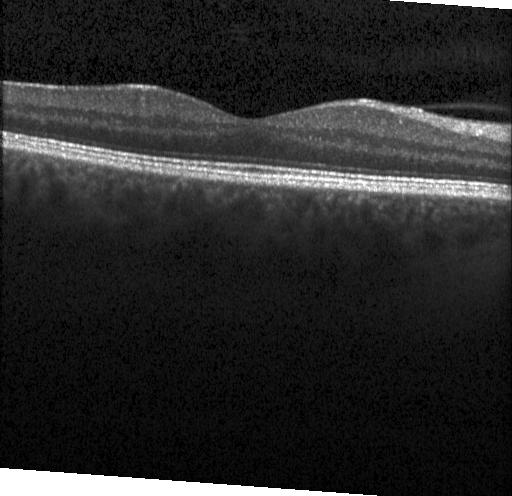

Finding: no choroidal neovascularization, no diabetic macular edema, and no drusen.